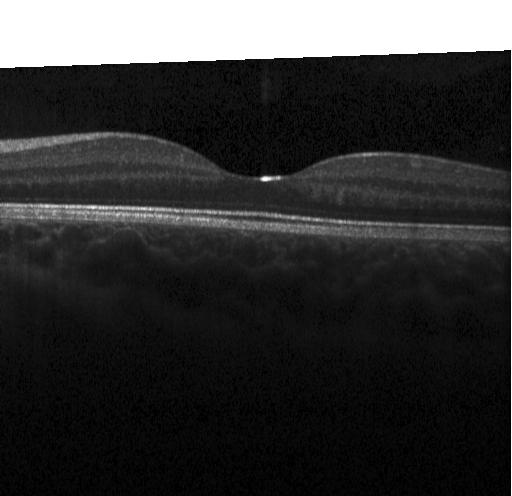

Optical coherence tomography B-scan; SD-OCT; instrument: Heidelberg Spectralis — This B-scan demonstrates no choroidal neovascularization, no diabetic macular edema, and no drusen.